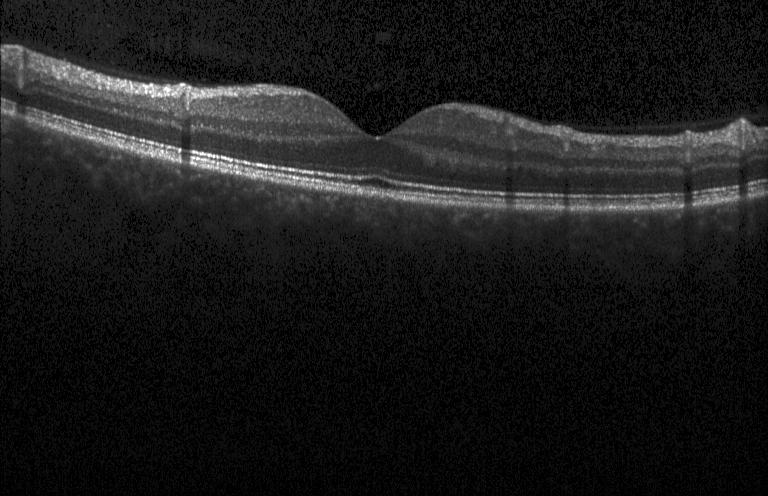
Instrument: Heidelberg Spectralis. Optical coherence tomography scan — Finding: no choroidal neovascularization, diabetic macular edema, or drusen.